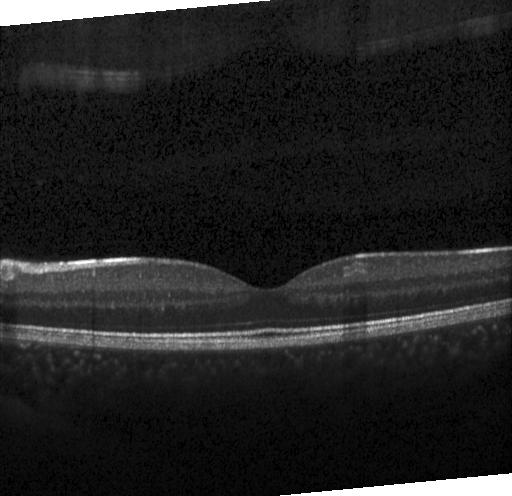

No choroidal neovascularization, no diabetic macular edema, and no drusen.